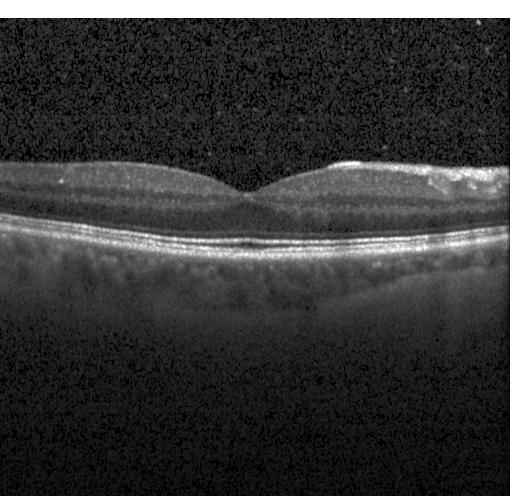 OCT finding: neither choroidal neovascularization, diabetic macular edema, nor drusen.